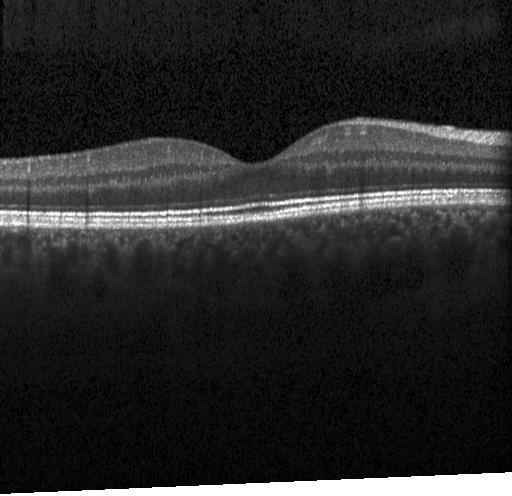 Centered on the fovea · optical coherence tomography scan · instrument: Heidelberg Spectralis · spectral-domain OCT
Diagnosis: neither choroidal neovascularization, diabetic macular edema, nor drusen.